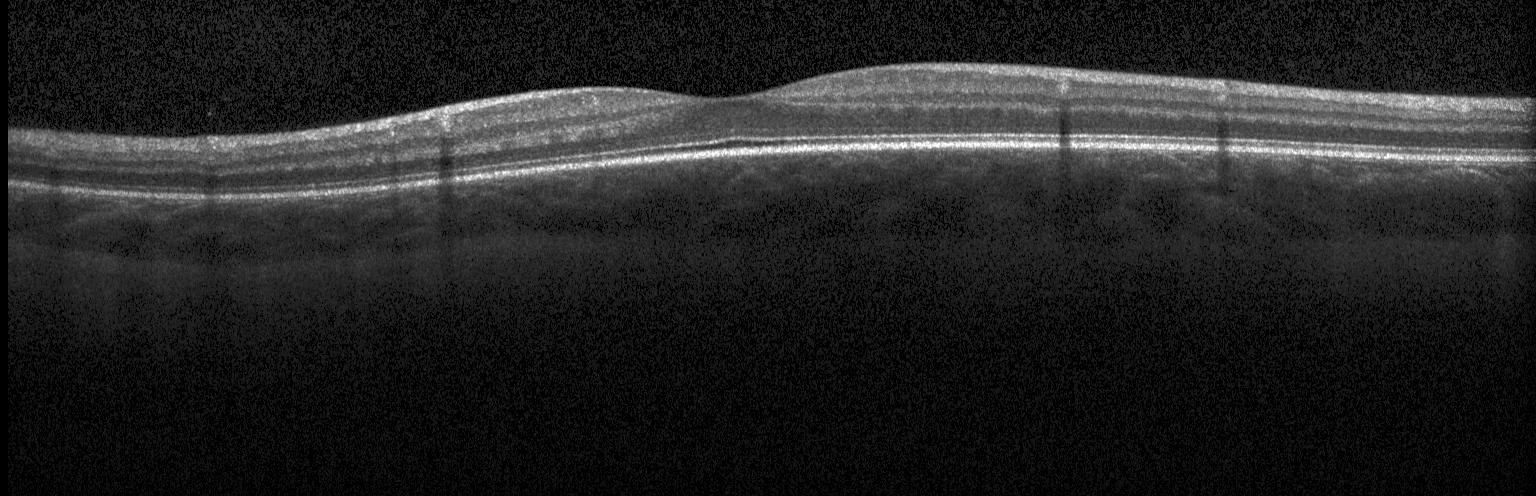 Heidelberg Spectralis OCT system · SD-OCT · retinal OCT cross-section. Diagnosis: no choroidal neovascularization, diabetic macular edema, or drusen.